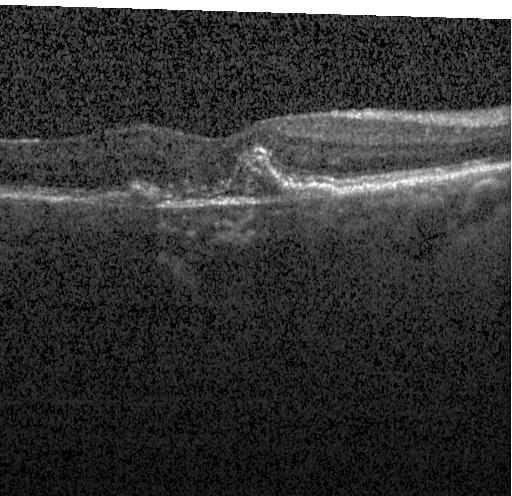 Impression: a choroidal neovascular membrane.